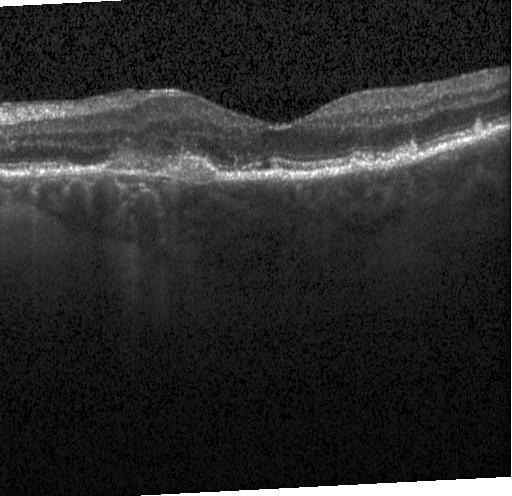
Heidelberg Spectralis. Horizontal scan through the fovea. SD-OCT. Retinal OCT B-scan
OCT finding: a choroidal neovascular membrane.